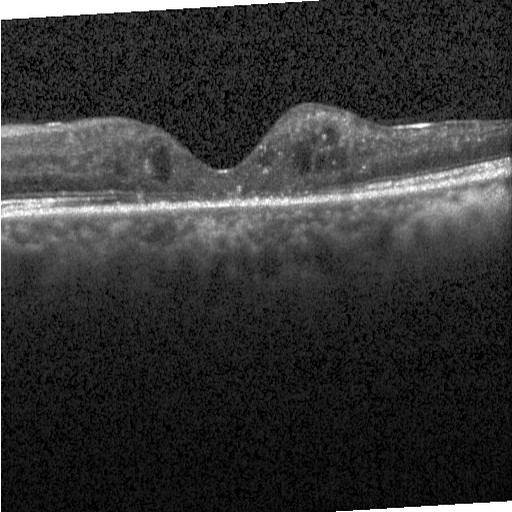
Acquired on a Heidelberg Spectralis, optical coherence tomography B-scan, macular scan
Impression: diabetic macular edema.